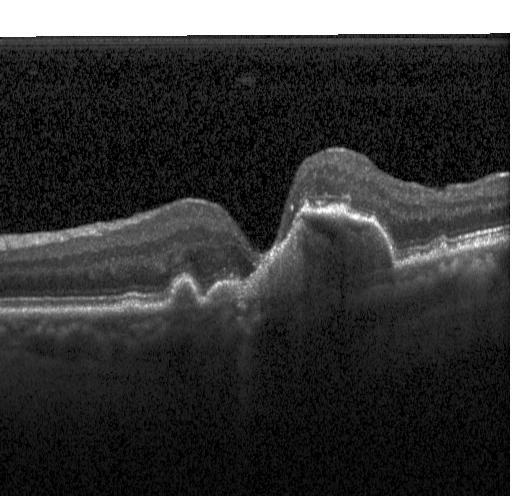

OCT B-scan · spectral-domain OCT
Impression: CNV.